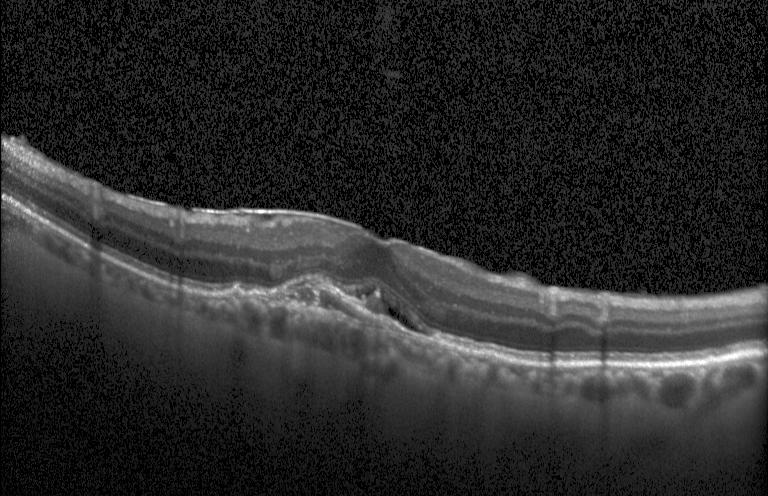
Dx: choroidal neovascularization (CNV).